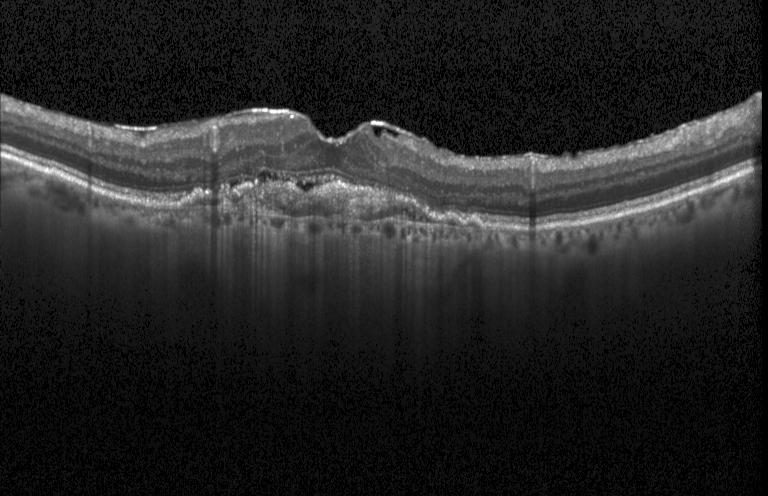 Dx: a choroidal neovascular membrane.